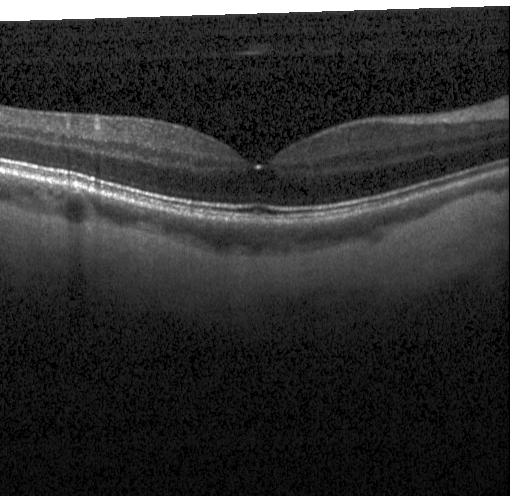 Optical coherence tomography B-scan — No evidence of choroidal neovascularization, diabetic macular edema, or drusen.